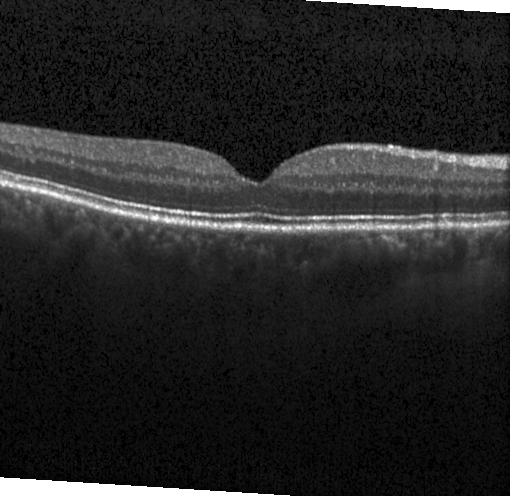 Retinal OCT cross-section
Diagnosis: no CNV, DME, or drusen.